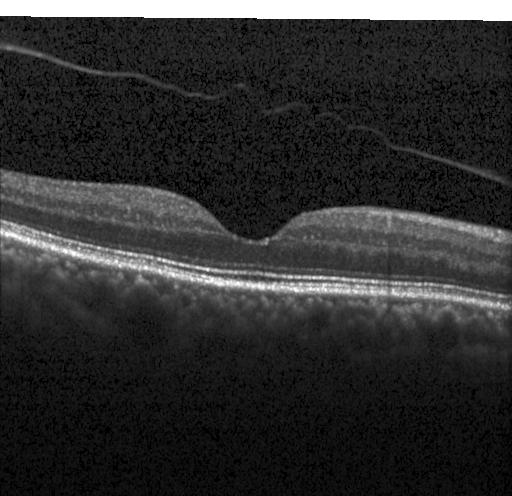 Diagnosis: no evidence of CNV, DME, or drusen.